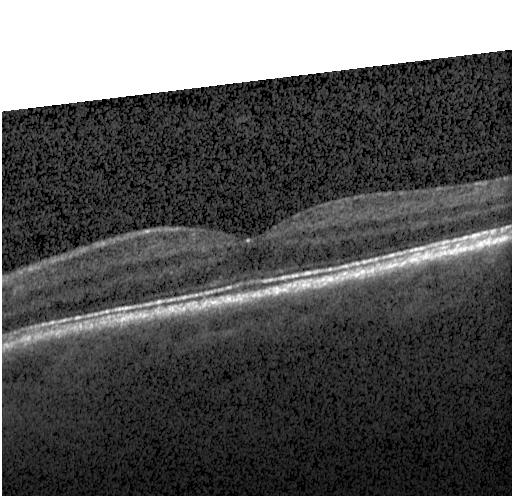

Impression: no choroidal neovascularization, diabetic macular edema, or drusen.